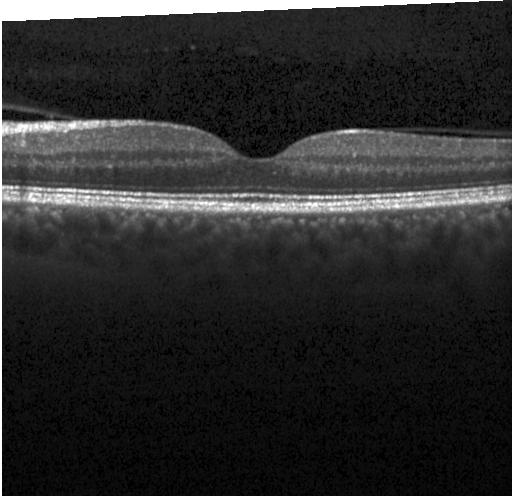 Finding: no evidence of CNV, DME, or drusen.